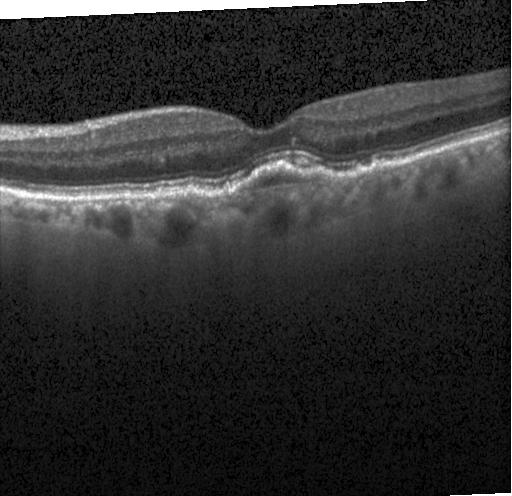

Impression: CNV.